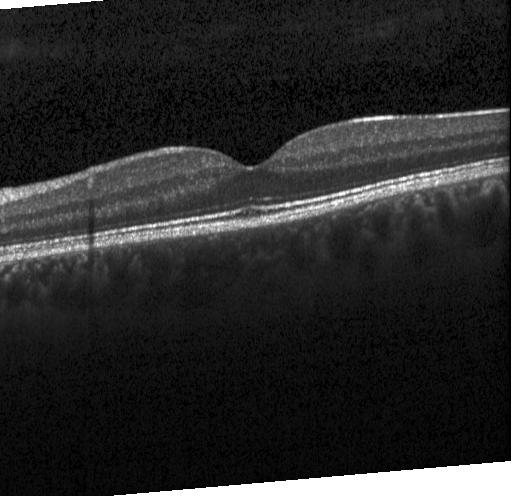
Macular OCT: no choroidal neovascularization, no diabetic macular edema, and no drusen.